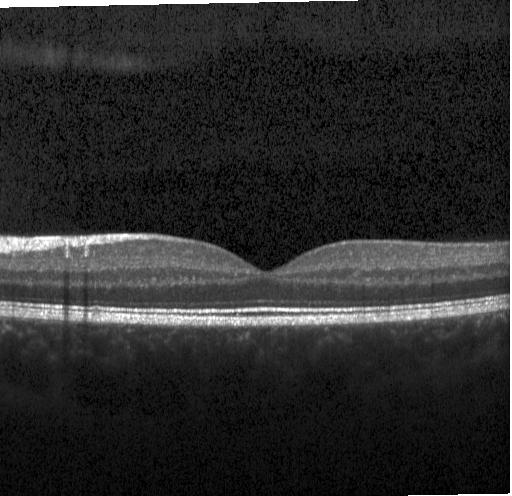

Retinal OCT cross-section showing no choroidal neovascularization, diabetic macular edema, or drusen.